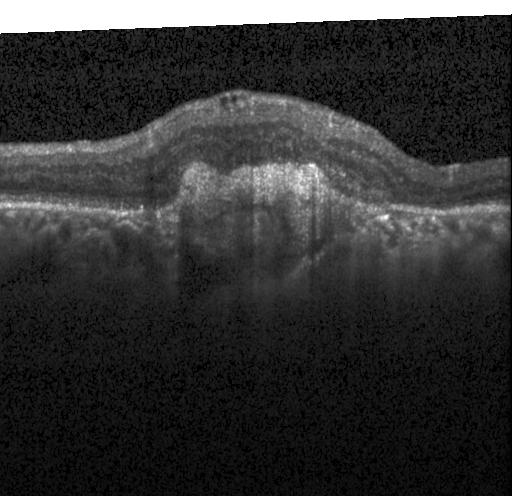

Macular OCT demonstrating a choroidal neovascular membrane.